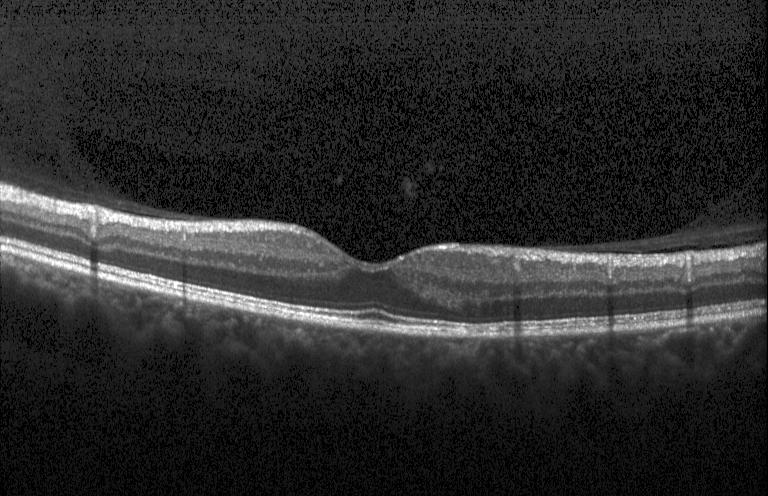

Retinal OCT B-scan · through the macula · instrument: Heidelberg Spectralis · spectral-domain optical coherence tomography. Impression: no choroidal neovascularization, diabetic macular edema, or drusen.